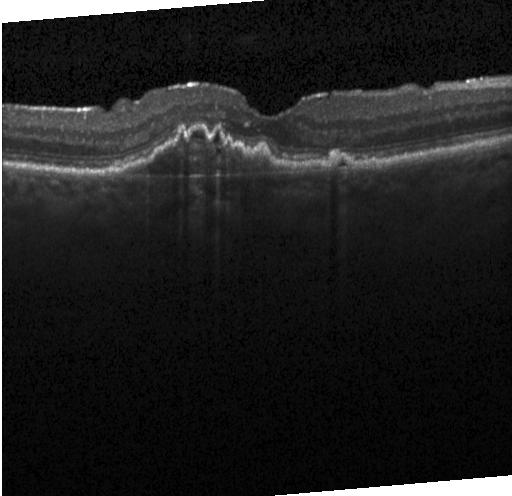

Retinal OCT cross-section; horizontal scan through the fovea; acquired on a Heidelberg Spectralis; SD-OCT — Diagnosis: a choroidal neovascular membrane.